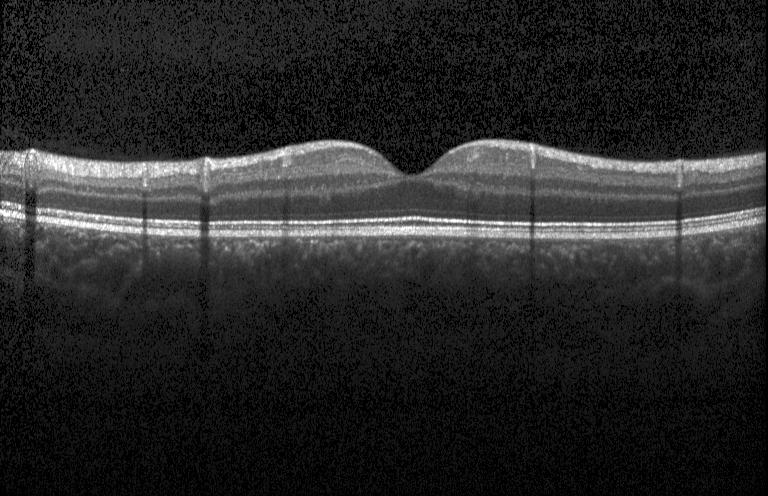
Retinal OCT B-scan. The scan shows no evidence of choroidal neovascularization, diabetic macular edema, or drusen.